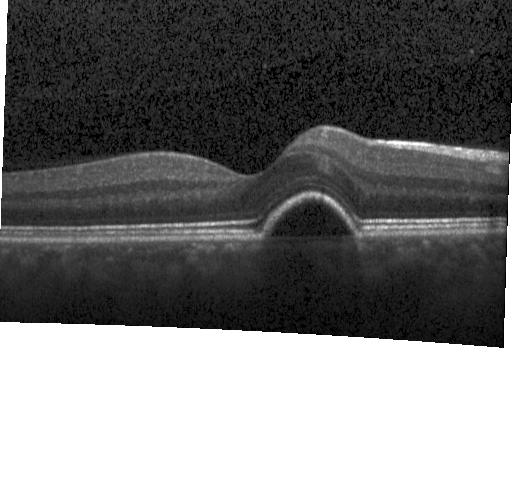
SD-OCT · retinal OCT B-scan · macular scan · Heidelberg Spectralis.
Finding: a choroidal neovascular membrane.